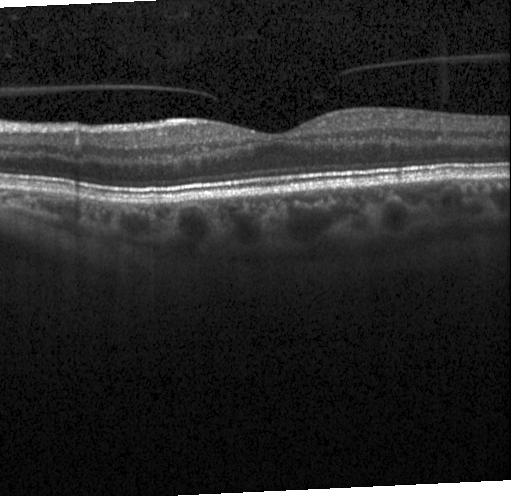
Optical coherence tomography scan
Diagnosis: no choroidal neovascularization, no diabetic macular edema, and no drusen.